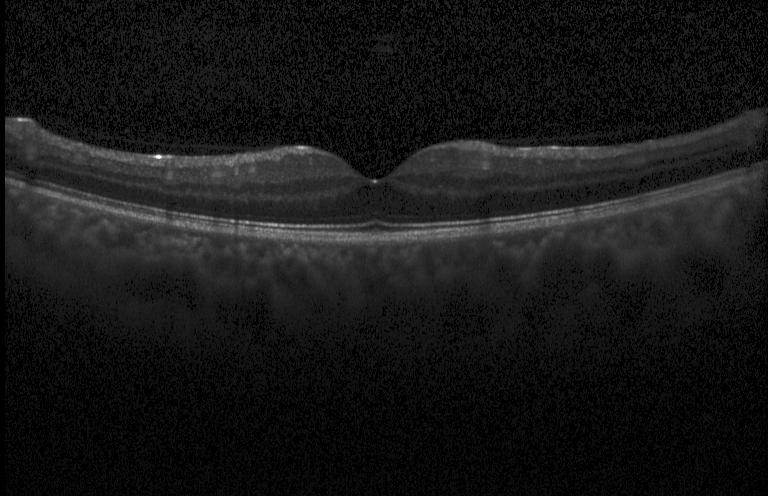
Assessment: no choroidal neovascularization, diabetic macular edema, or drusen.